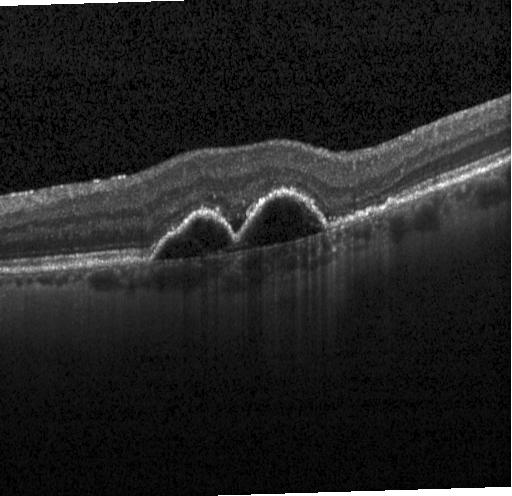

The scan shows a choroidal neovascular membrane.